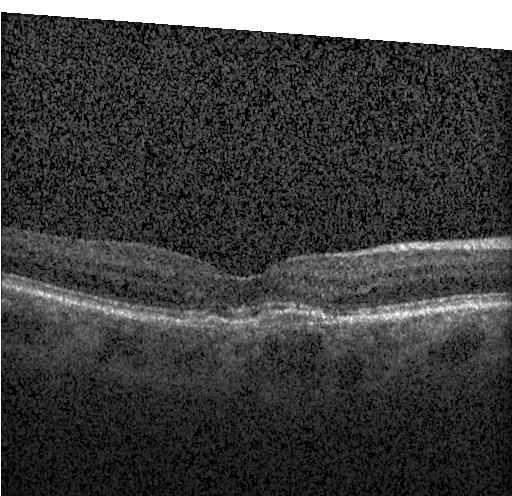 OCT B-scan — Dx: a choroidal neovascular membrane.